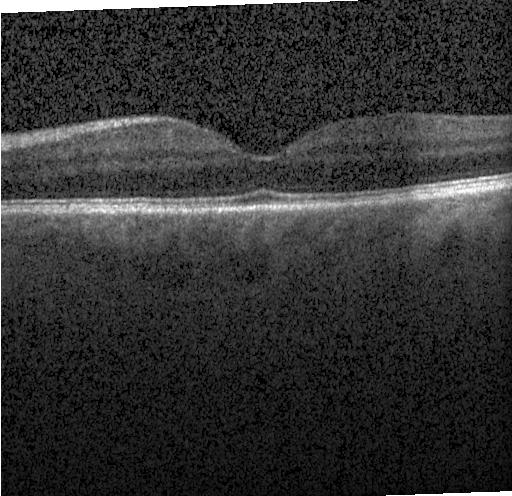 Impression: no evidence of choroidal neovascularization, diabetic macular edema, or drusen.